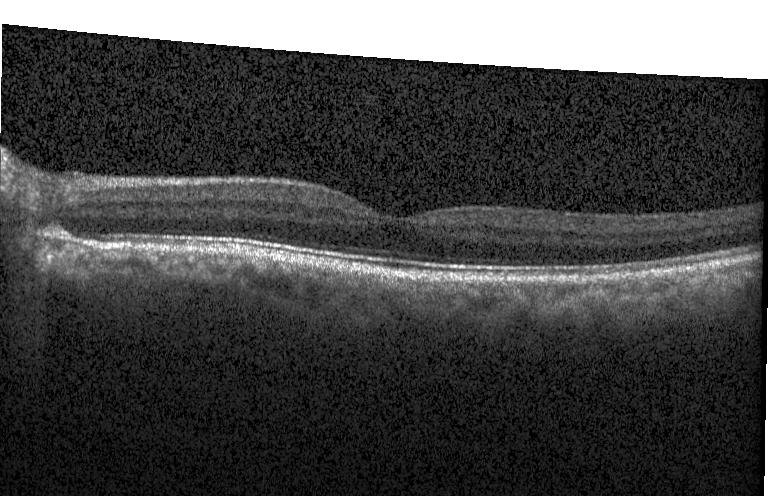

Retinal OCT cross-section showing no choroidal neovascularization, no diabetic macular edema, and no drusen.